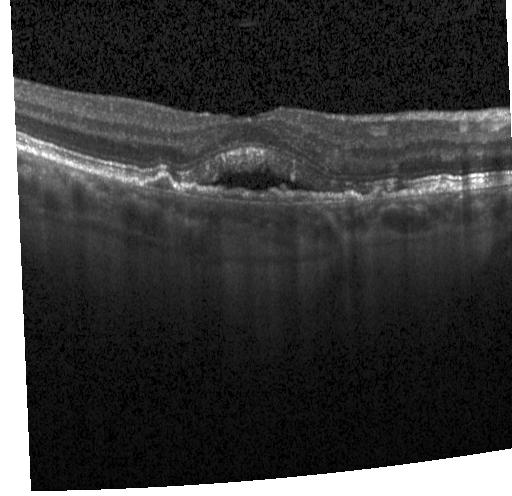 Horizontal scan through the fovea. OCT line scan.
This B-scan demonstrates a choroidal neovascular membrane.